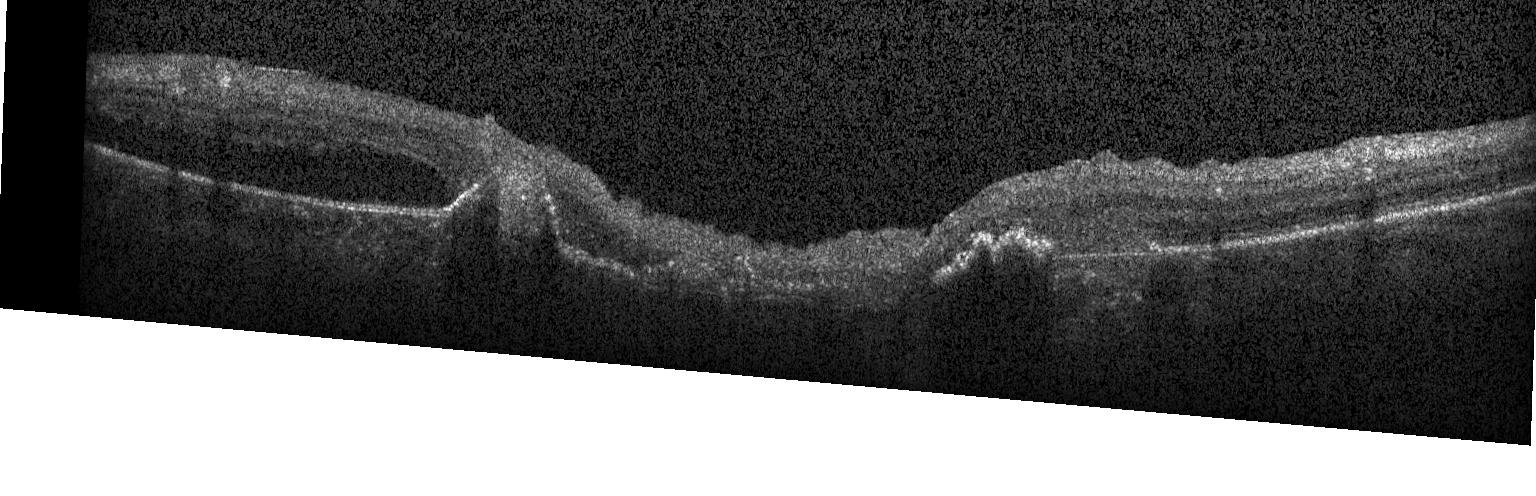 Retinal OCT B-scan · Heidelberg Spectralis OCT system. Assessment: a choroidal neovascular membrane.